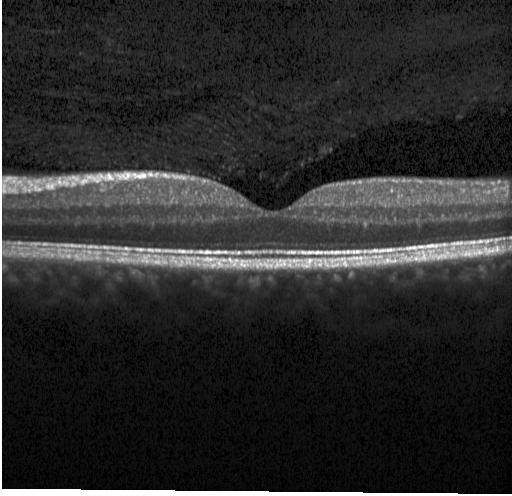

No CNV, DME, or drusen.